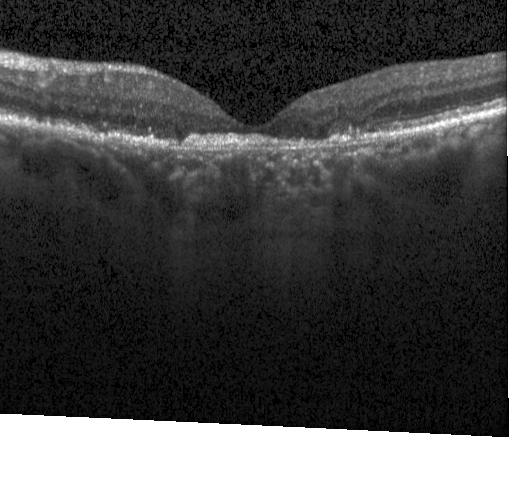
Optical coherence tomography B-scan · centered on the fovea — Finding: CNV.